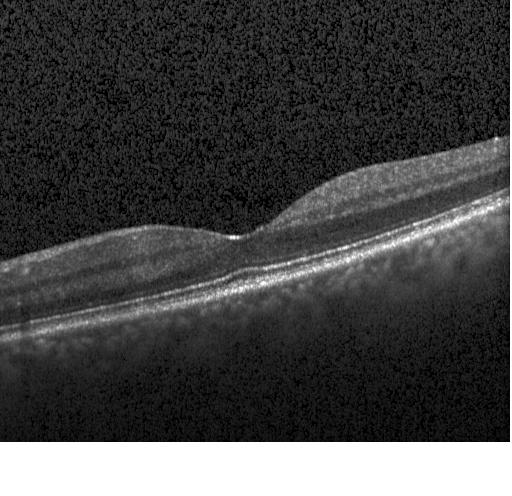

Retinal OCT B-scan.
This B-scan demonstrates no choroidal neovascularization, no diabetic macular edema, and no drusen.